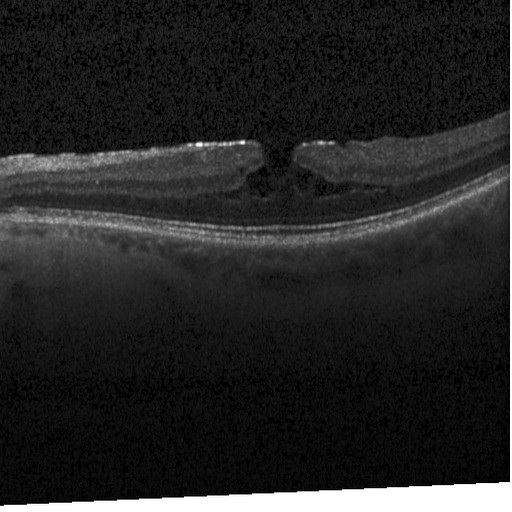
The scan shows diabetic macular edema.